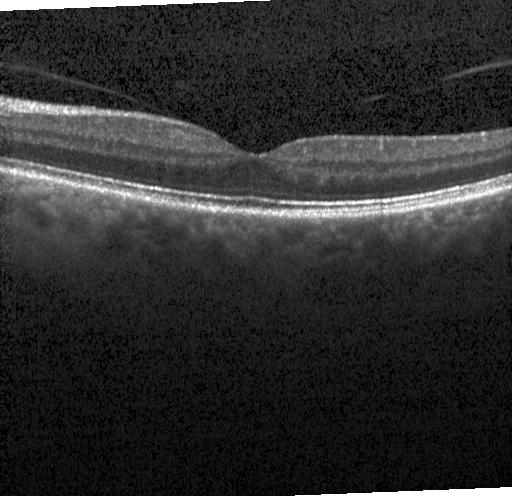
Heidelberg Spectralis OCT system · OCT B-scan · macular scan · spectral-domain OCT.
Diagnosis: no choroidal neovascularization, no diabetic macular edema, and no drusen.